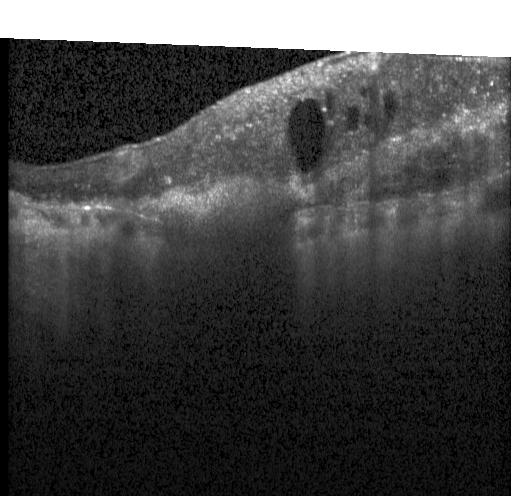 Finding: choroidal neovascularization.